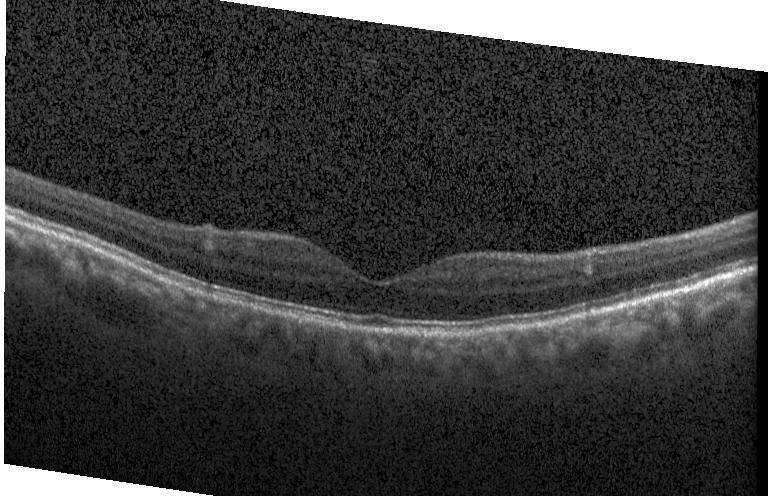

Optical coherence tomography scan
Neither choroidal neovascularization, diabetic macular edema, nor drusen.